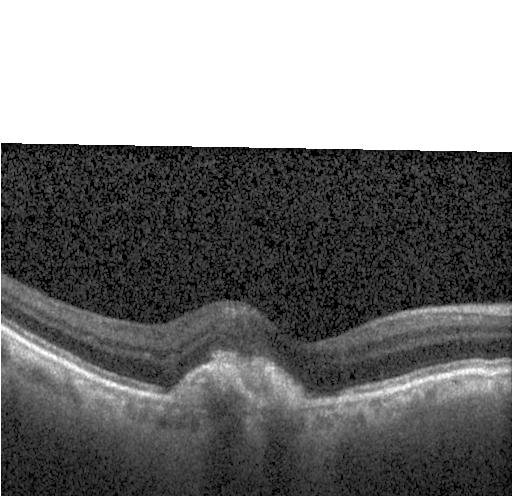
Spectral-domain optical coherence tomography, optical coherence tomography B-scan.
Impression: CNV.